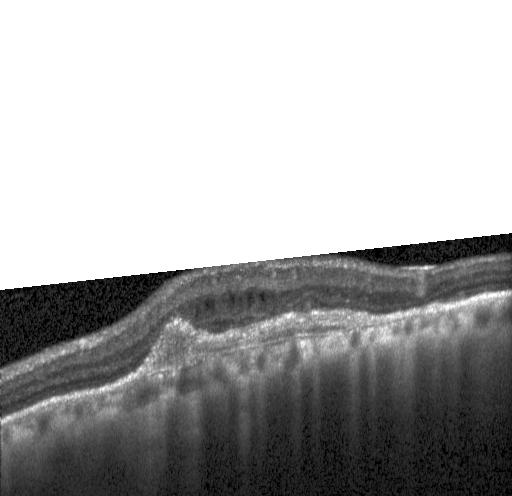

Diagnosis: CNV.